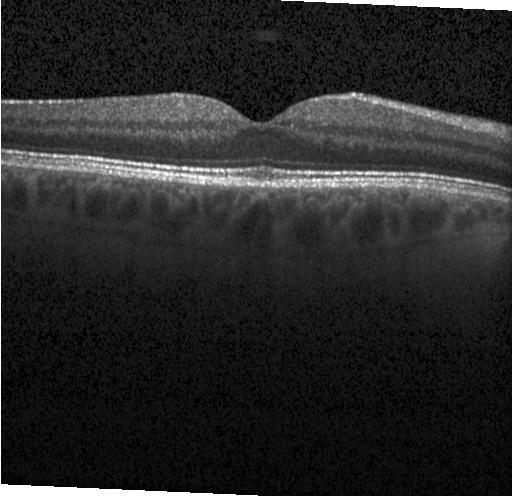

Optical coherence tomography scan, horizontal scan through the fovea, acquired on a Heidelberg Spectralis — This B-scan demonstrates no choroidal neovascularization, no diabetic macular edema, and no drusen.